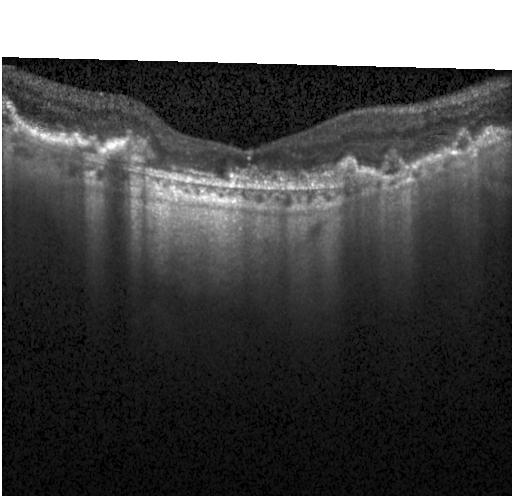

OCT finding: choroidal neovascularization (CNV).